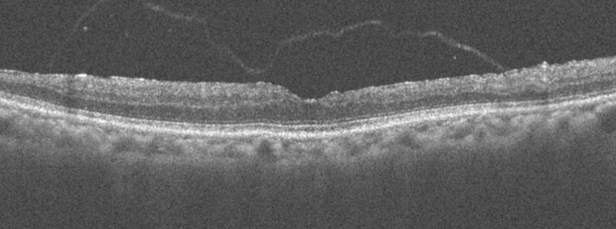
Retinal OCT cross-section; instrument: Optovue Avanti RTVue XR; through the macula. Finding: epiretinal membrane (ERM).